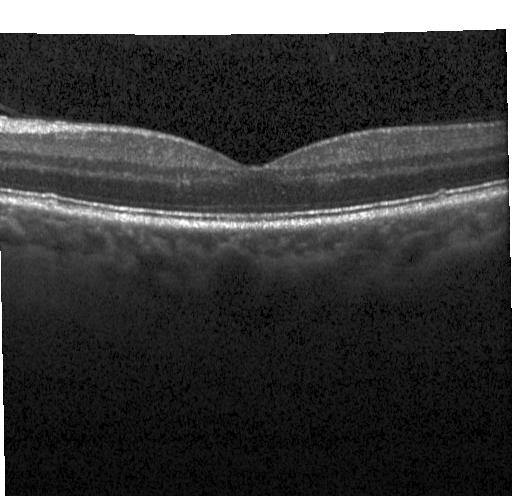
Optical coherence tomography B-scan — Finding: sub-RPE drusenoid deposits.